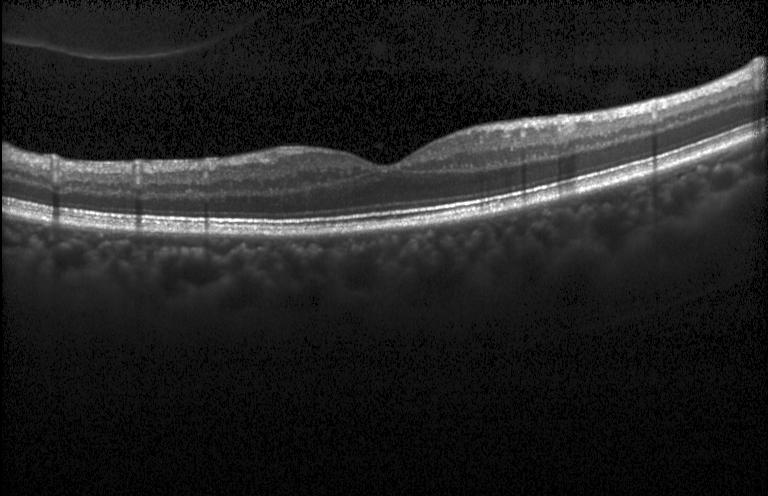 Horizontal scan through the fovea · OCT line scan — Diagnosis: no evidence of choroidal neovascularization, diabetic macular edema, or drusen.